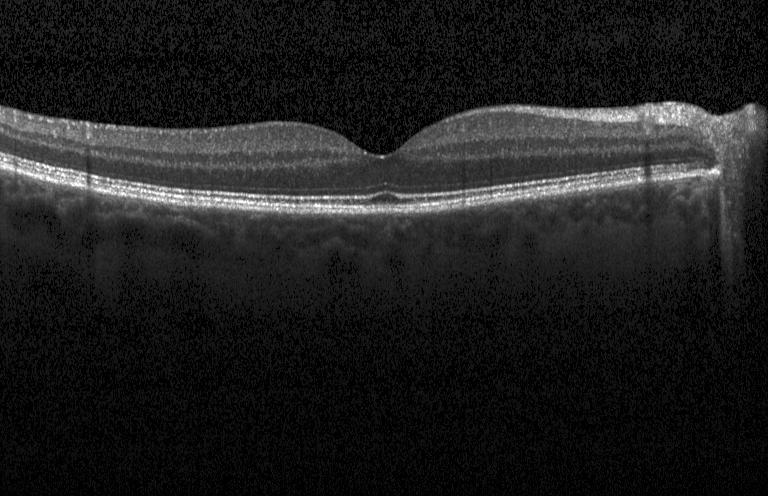 OCT line scan — Macular OCT: no CNV, DME, or drusen.